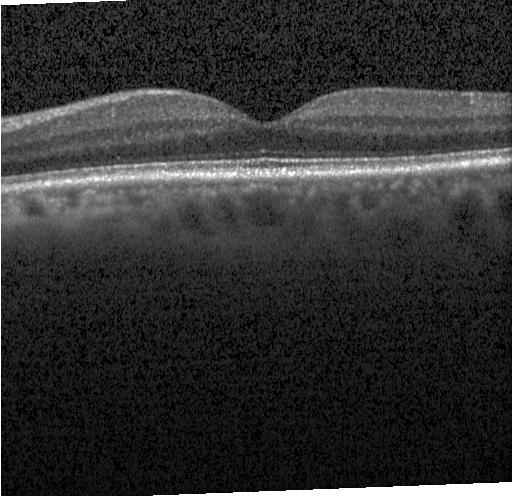

Impression: neither choroidal neovascularization, diabetic macular edema, nor drusen.